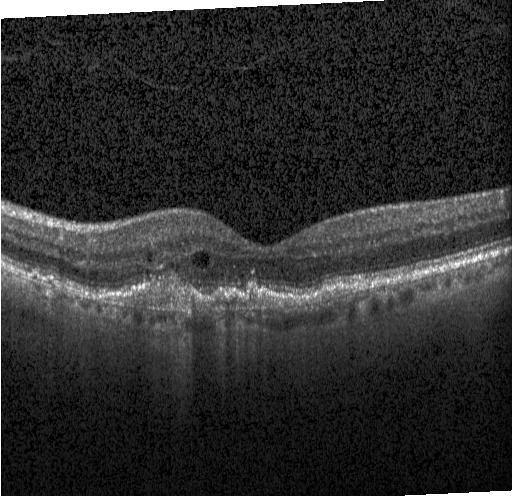 Assessment: a choroidal neovascular membrane.